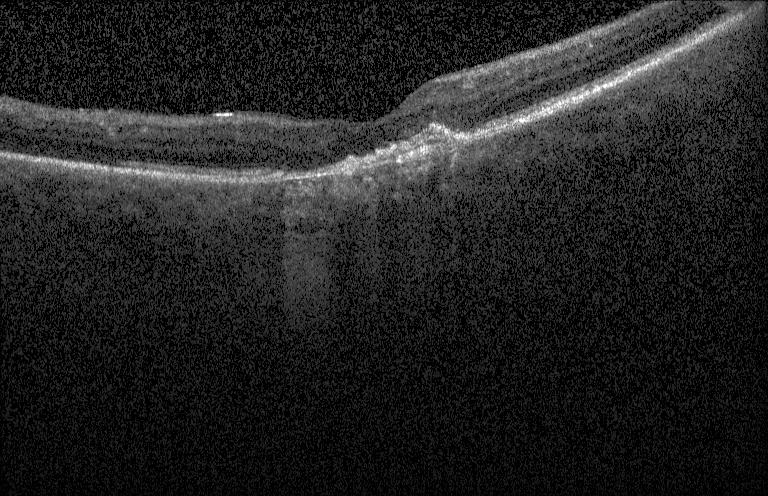
Diagnosis: a choroidal neovascular membrane.